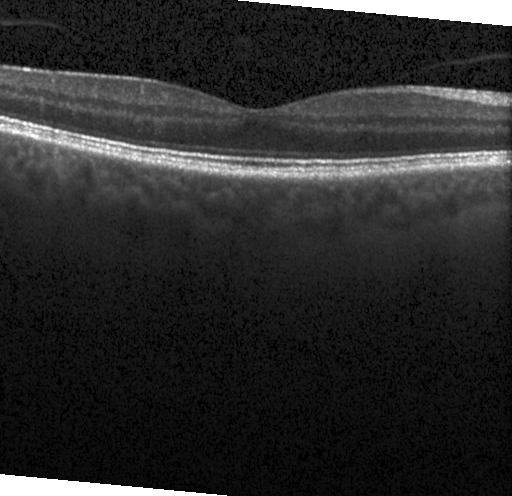 This B-scan demonstrates no choroidal neovascularization, diabetic macular edema, or drusen.